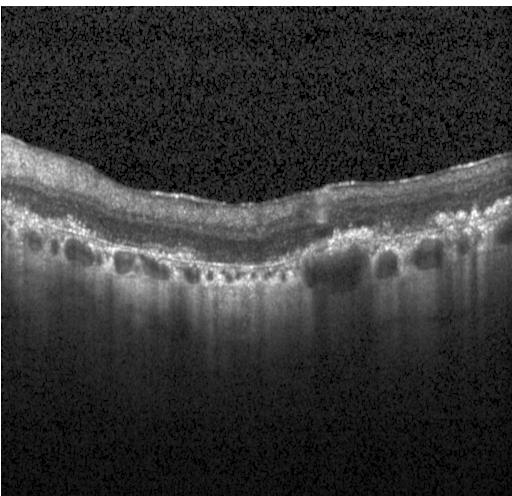
Retinal OCT B-scan · SD-OCT.
Impression: a choroidal neovascular membrane.